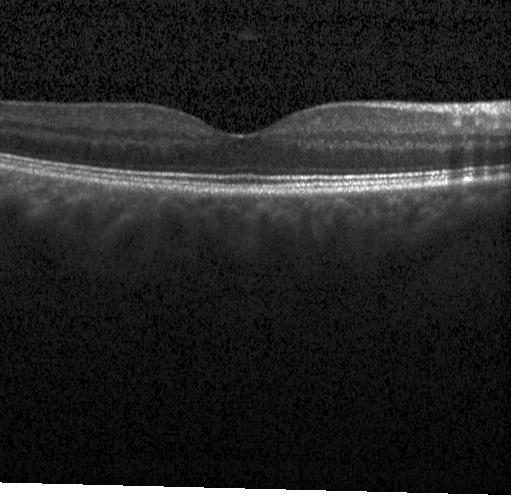

Finding: no choroidal neovascularization, no diabetic macular edema, and no drusen.